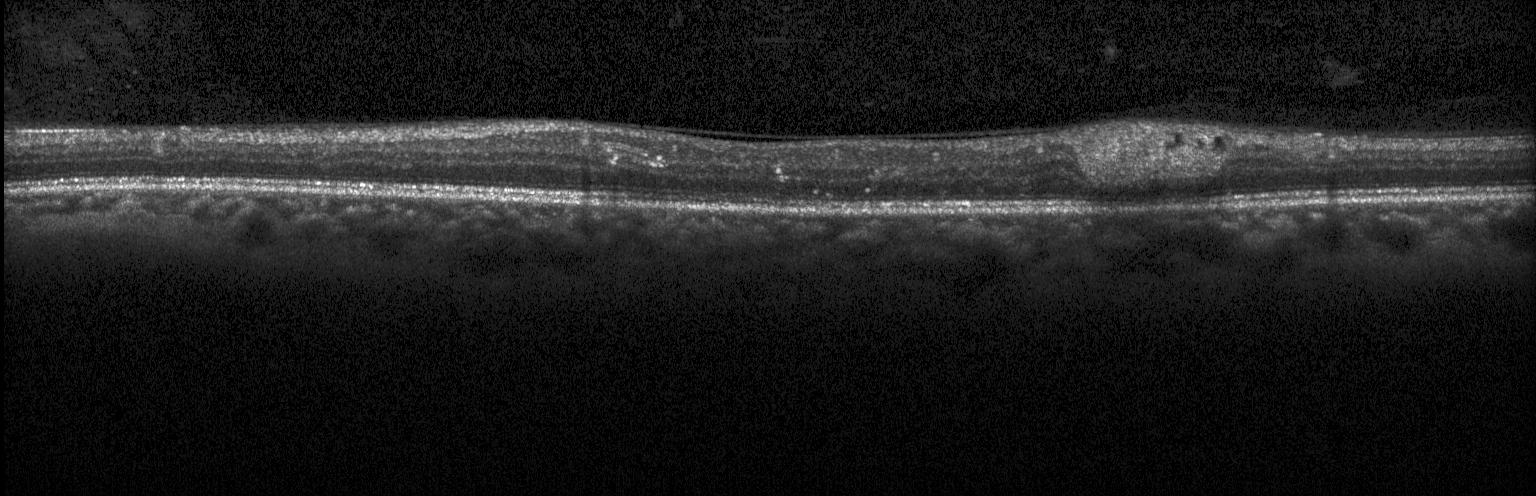

Macular OCT demonstrating diabetic macular edema (DME).